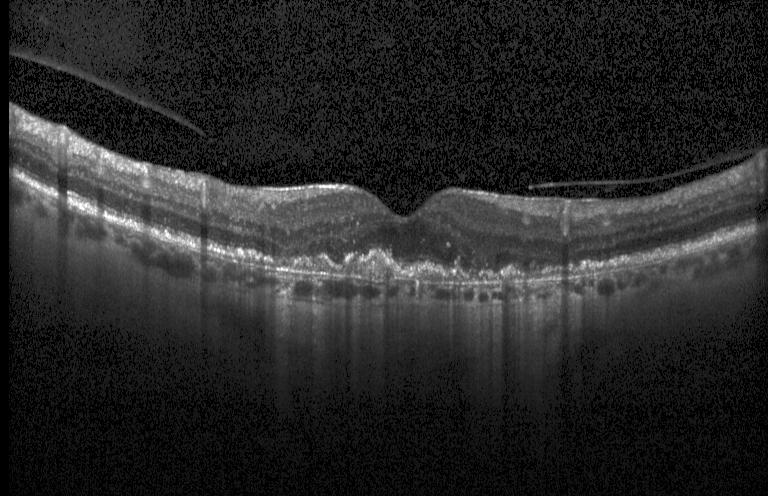

Optical coherence tomography B-scan. Impression: choroidal neovascularization (CNV).